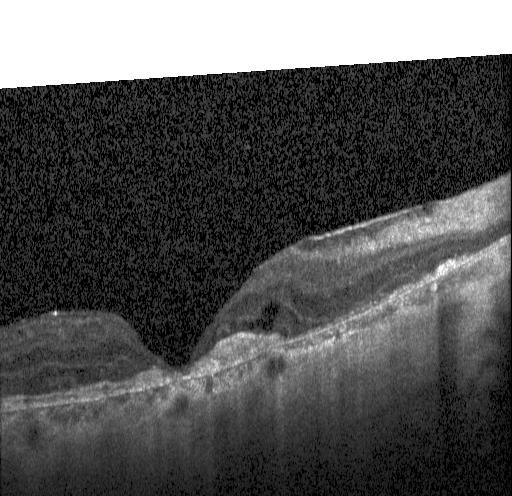 This B-scan demonstrates a choroidal neovascular membrane.